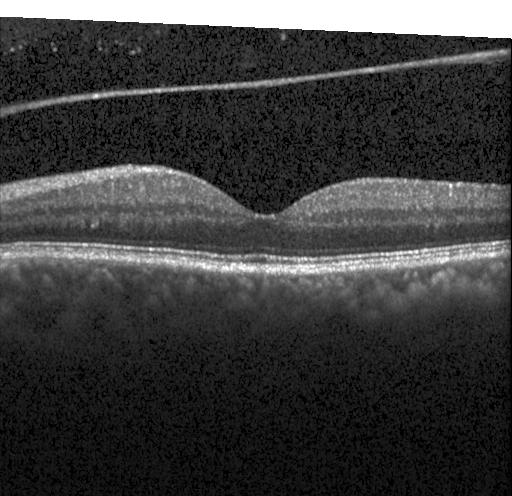
Heidelberg Spectralis OCT system, optical coherence tomography B-scan, spectral-domain optical coherence tomography — Finding: neither choroidal neovascularization, diabetic macular edema, nor drusen.